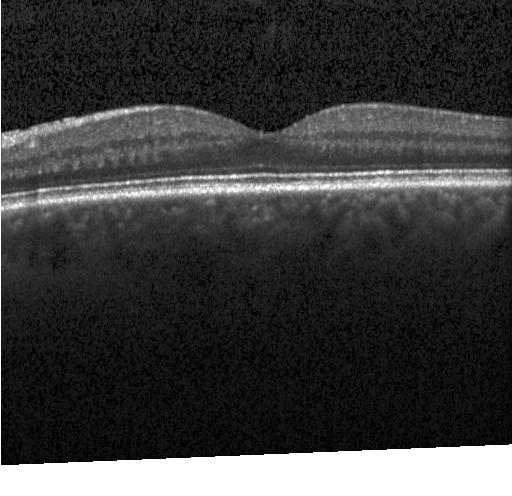

Optical coherence tomography B-scan. Instrument: Heidelberg Spectralis. Centered on the fovea. SD-OCT — Assessment: no evidence of CNV, DME, or drusen.